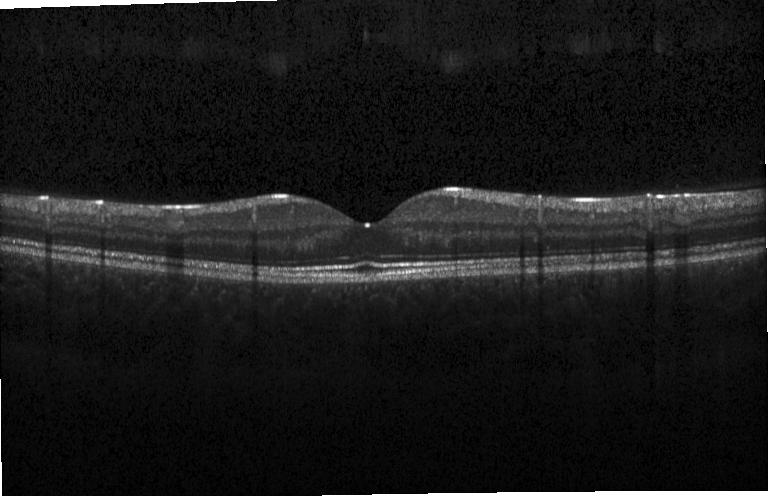
Retinal OCT cross-section showing no evidence of choroidal neovascularization, diabetic macular edema, or drusen.